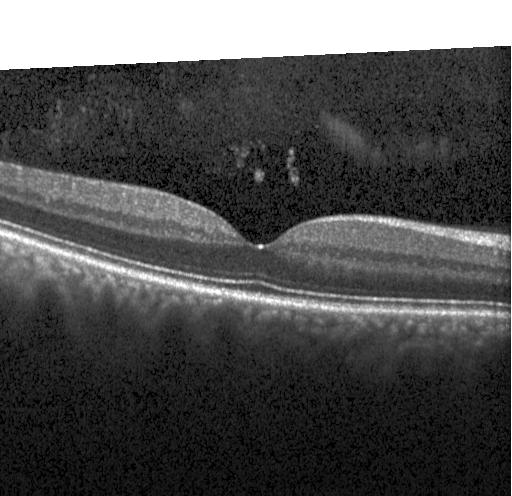
The scan shows no choroidal neovascularization, no diabetic macular edema, and no drusen.